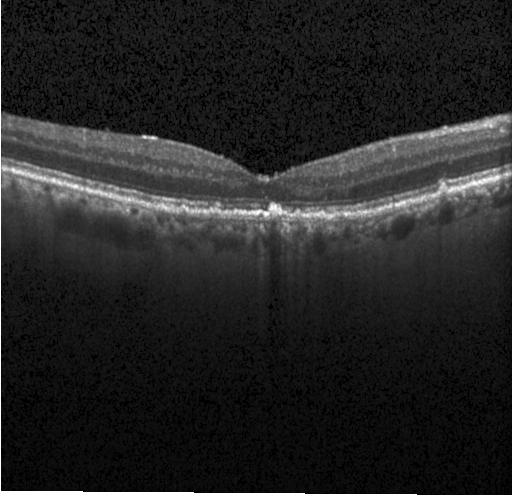

Horizontal scan through the fovea. Optical coherence tomography B-scan. Heidelberg Spectralis. Spectral-domain optical coherence tomography — Diagnosis: drusen.